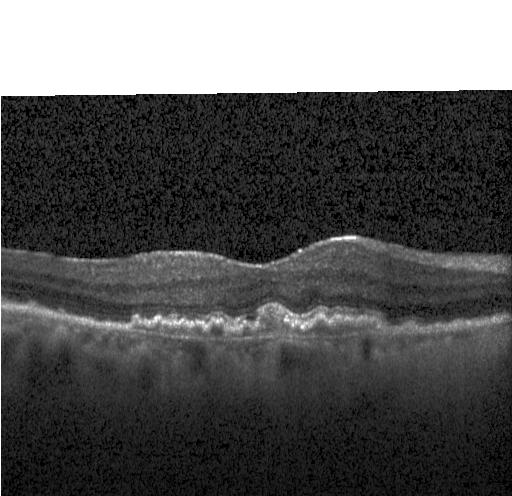 The scan shows choroidal neovascularization (CNV).